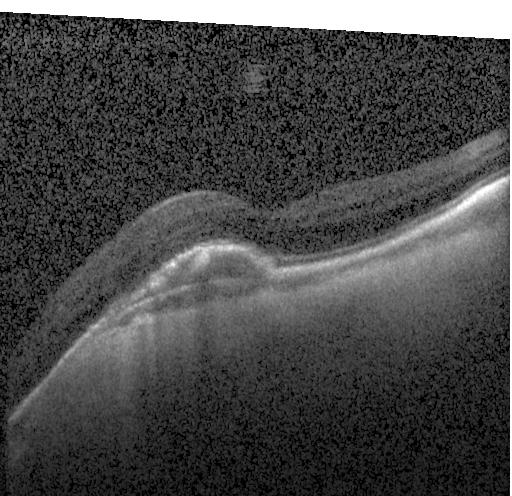

Diagnosis: a choroidal neovascular membrane.